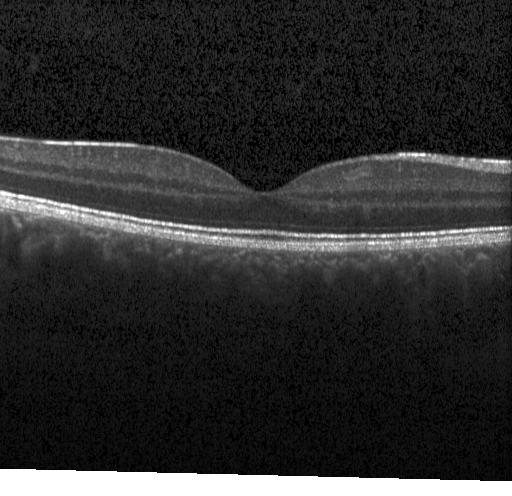

Optical coherence tomography scan. Finding: no evidence of choroidal neovascularization, diabetic macular edema, or drusen.